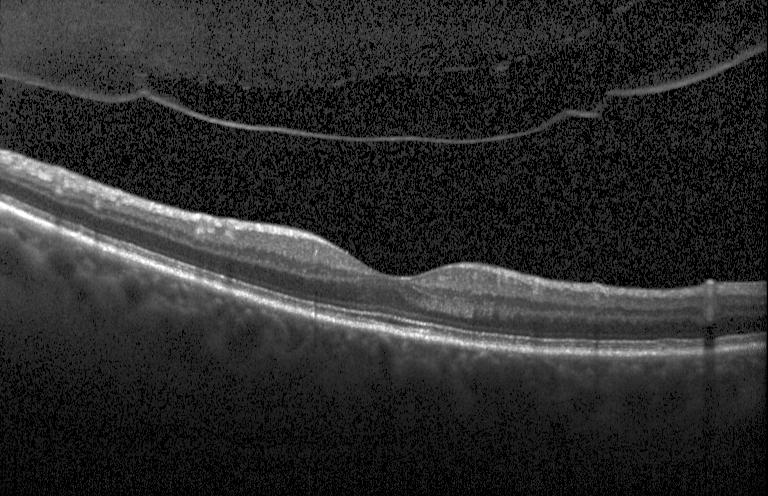
Instrument: Heidelberg Spectralis; OCT B-scan. Diagnosis: no CNV, DME, or drusen.